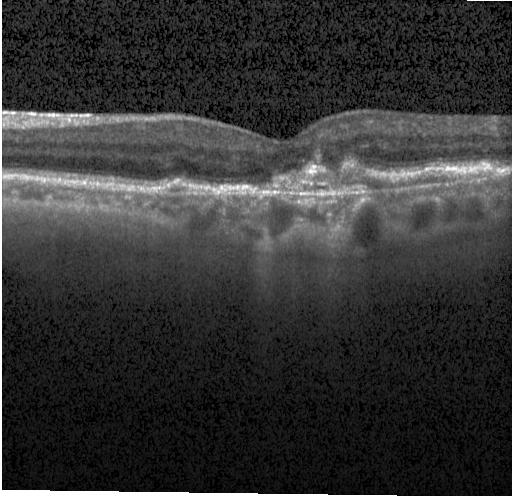 OCT finding: a choroidal neovascular membrane.